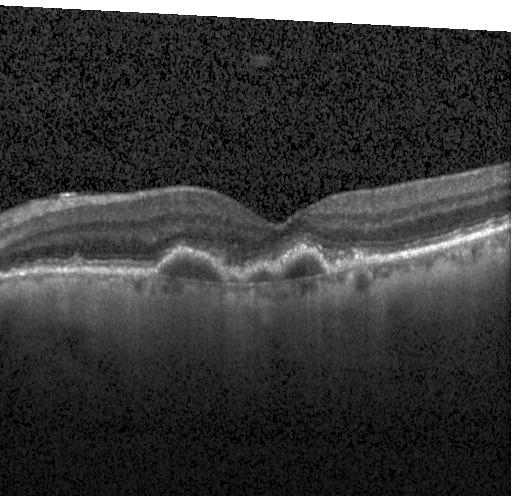 Macular OCT: CNV.